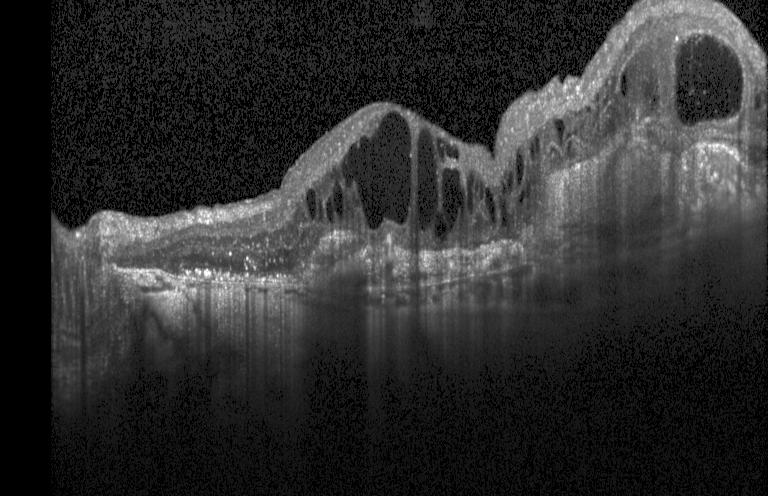

Impression: choroidal neovascularization.